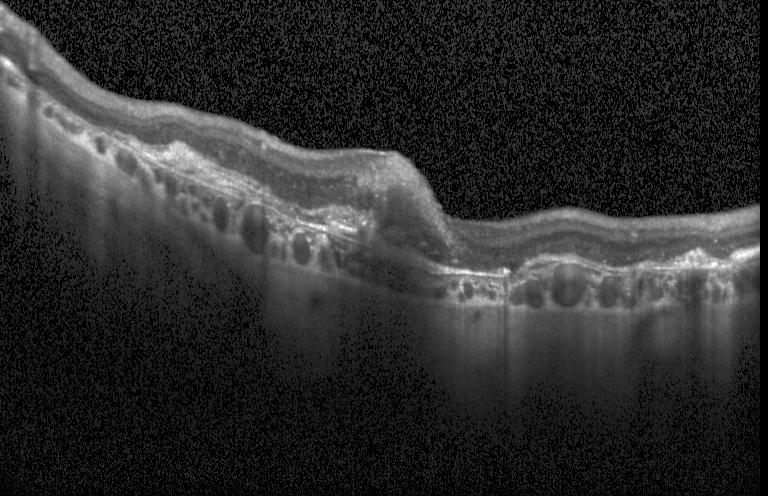 Centered on the fovea, OCT B-scan
A choroidal neovascular membrane.